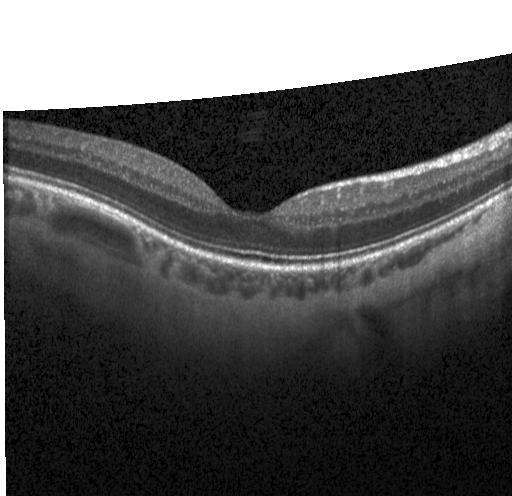

OCT B-scan showing neither choroidal neovascularization, diabetic macular edema, nor drusen.